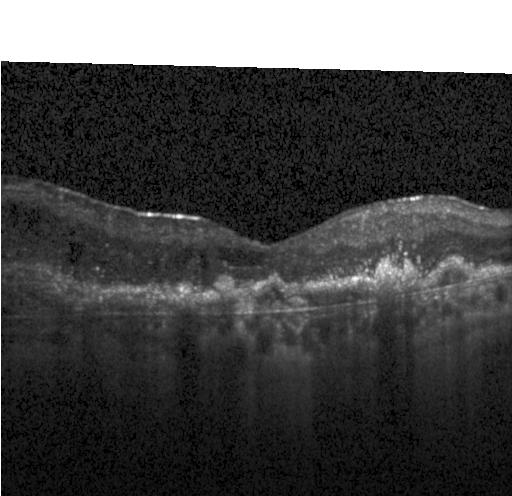

Centered on the fovea · acquired on a Heidelberg Spectralis · retinal OCT B-scan · SD-OCT
Diagnosis: CNV.